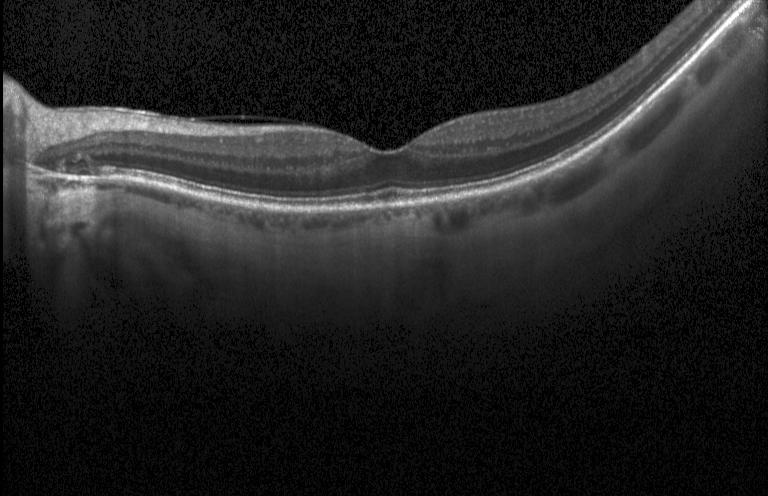 Optical coherence tomography B-scan
Neither choroidal neovascularization, diabetic macular edema, nor drusen.